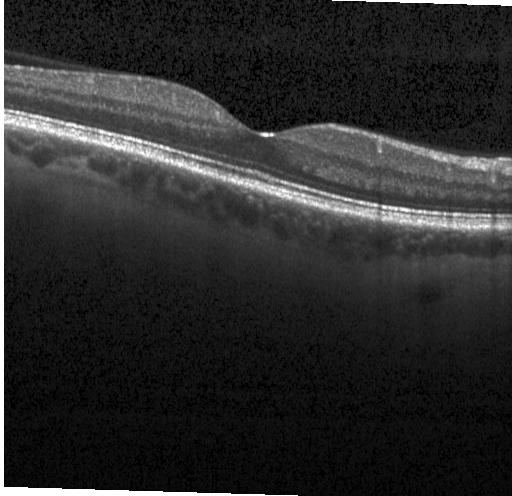 Centered on the fovea, Heidelberg Spectralis, retinal OCT cross-section — Diagnosis: neither choroidal neovascularization, diabetic macular edema, nor drusen.